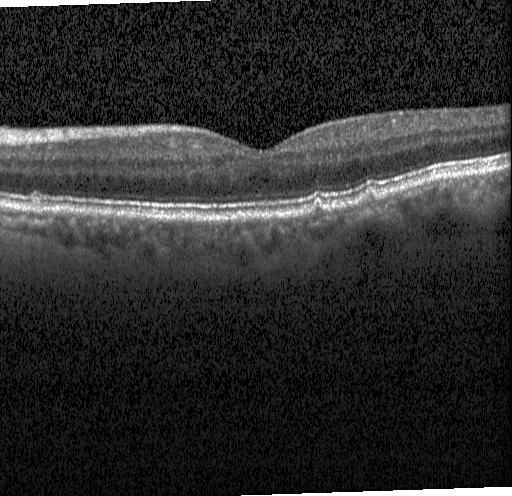 Acquired on a Heidelberg Spectralis · SD-OCT · macular scan · OCT B-scan — Finding: multiple drusen.